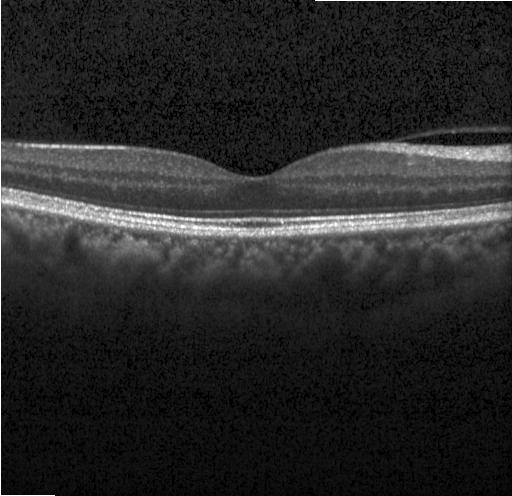 OCT line scan, instrument: Heidelberg Spectralis.
OCT finding: no CNV, DME, or drusen.